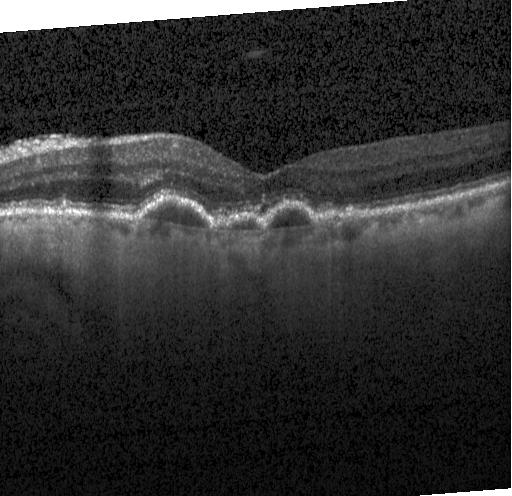 Retinal OCT B-scan, Heidelberg Spectralis
The scan shows a choroidal neovascular membrane.